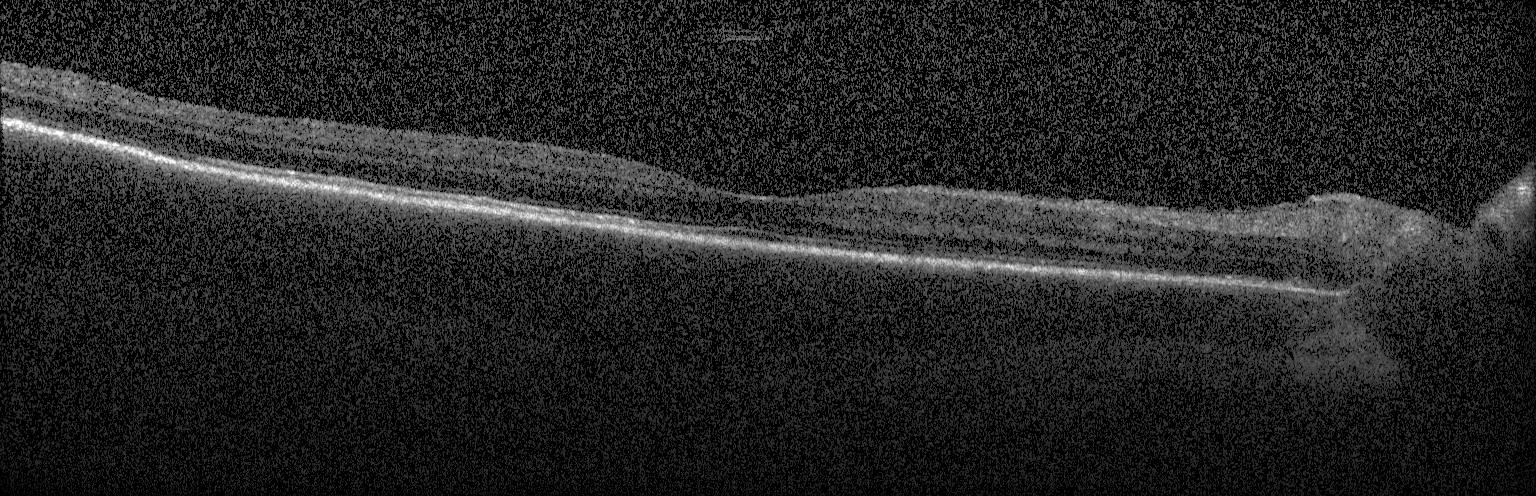 OCT B-scan — Diagnosis: no CNV, no DME, and no drusen.